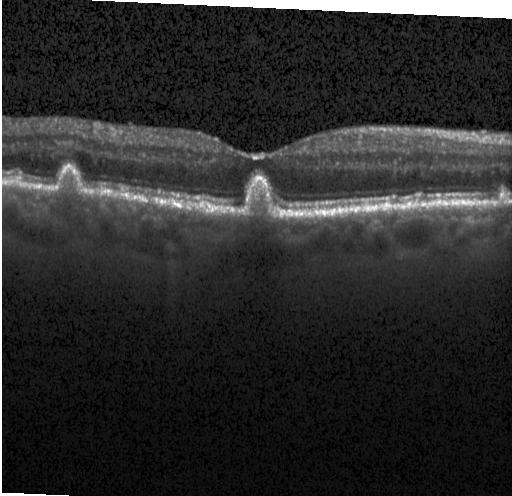

Horizontal scan through the fovea. Optical coherence tomography B-scan. Instrument: Heidelberg Spectralis. Finding: drusen.